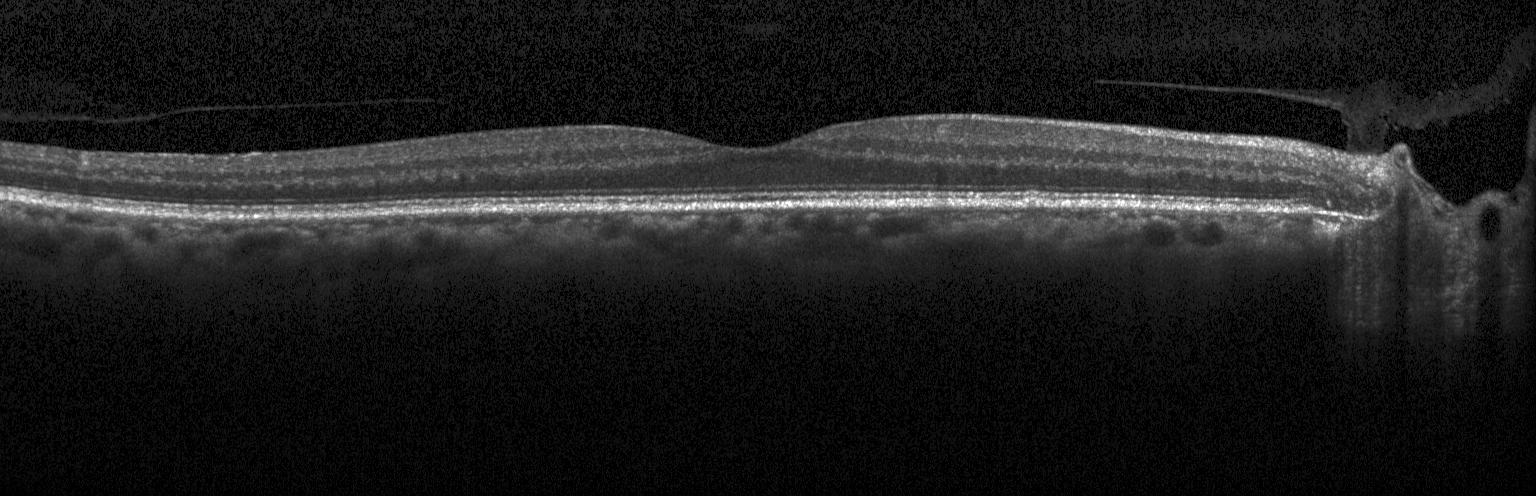

Spectral-domain optical coherence tomography, instrument: Heidelberg Spectralis, fovea-centered, OCT line scan — Diagnosis: neither choroidal neovascularization, diabetic macular edema, nor drusen.